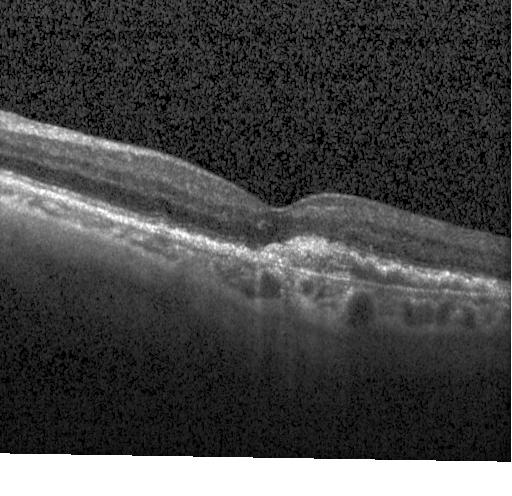 Spectral-domain OCT · instrument: Heidelberg Spectralis · retinal OCT B-scan. OCT finding: a choroidal neovascular membrane.